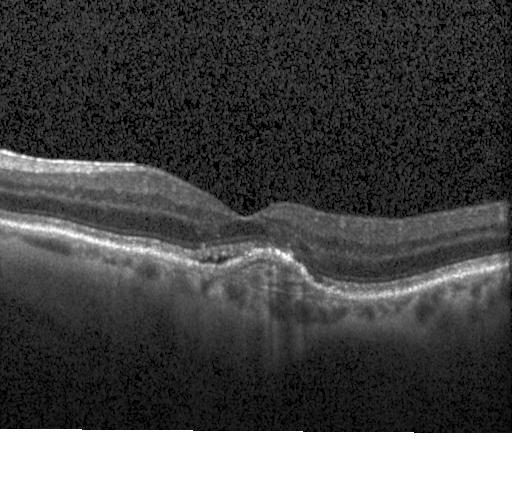 Impression: choroidal neovascularization.